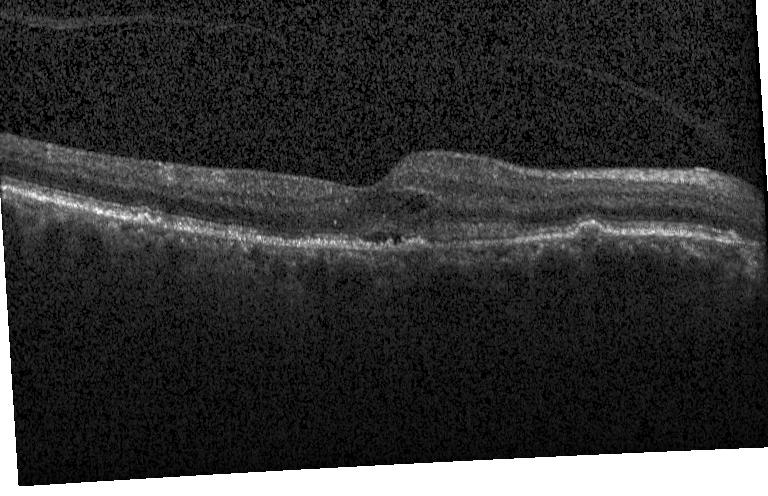

OCT line scan. Fovea-centered.
Impression: choroidal neovascularization.